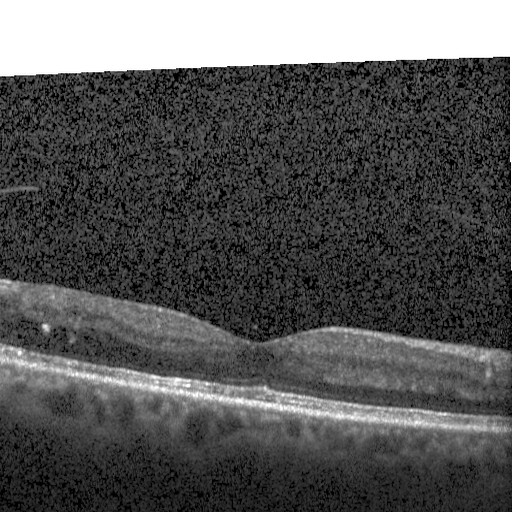
Optical coherence tomography scan — Diagnosis: DME.